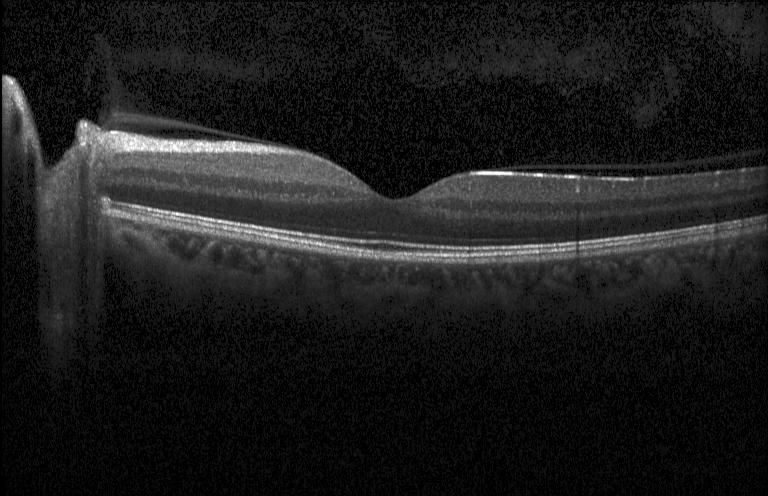 Retinal OCT cross-section — Macular OCT: no evidence of choroidal neovascularization, diabetic macular edema, or drusen.